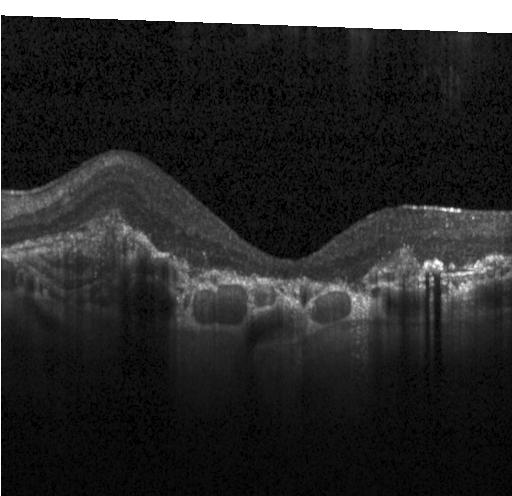 OCT B-scan
Diagnosis: a choroidal neovascular membrane.